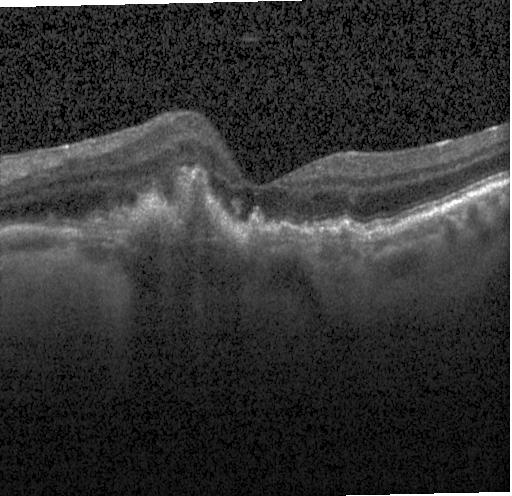 OCT B-scan, acquired on a Heidelberg Spectralis, spectral-domain optical coherence tomography, centered on the fovea
Finding: a choroidal neovascular membrane.